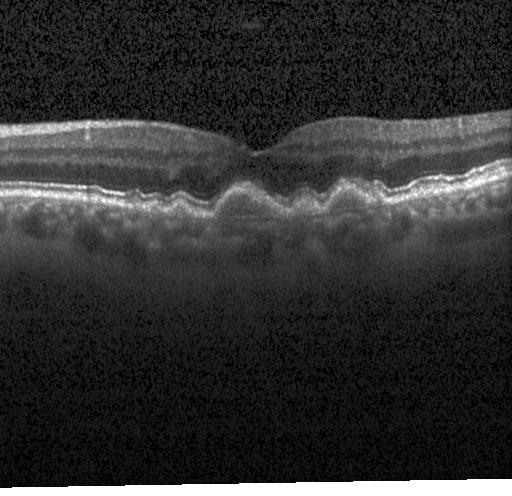

Macular OCT demonstrating sub-RPE drusenoid deposits.